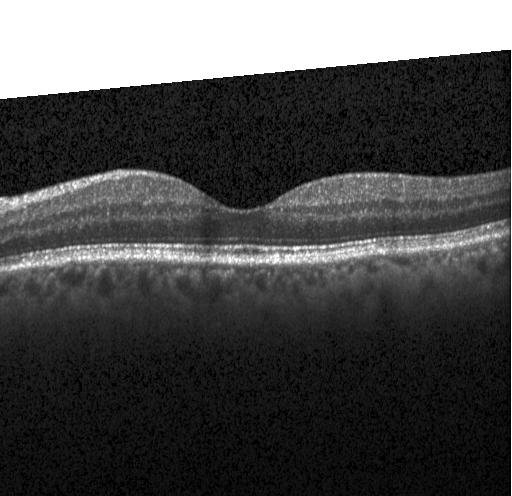 Retinal OCT cross-section, centered on the fovea, acquired on a Heidelberg Spectralis
This B-scan demonstrates no CNV, DME, or drusen.